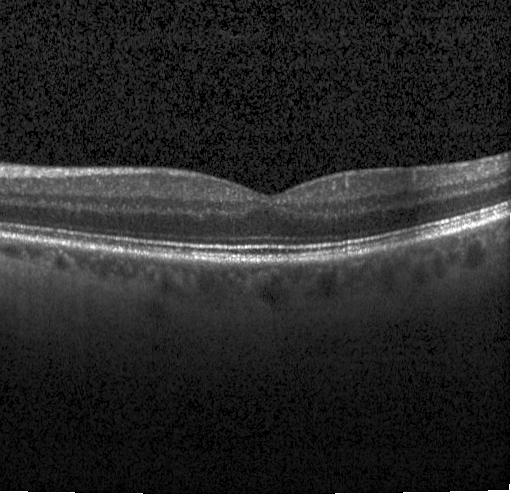

Impression: no evidence of choroidal neovascularization, diabetic macular edema, or drusen.